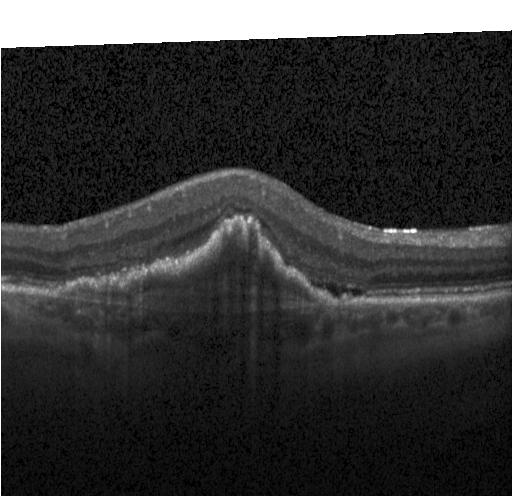

The scan shows a choroidal neovascular membrane.